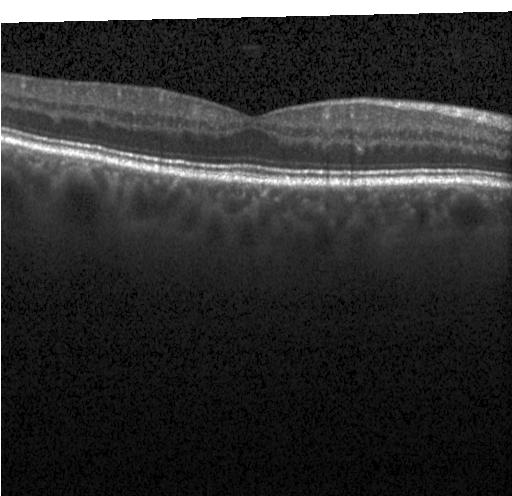

OCT scan showing no evidence of choroidal neovascularization, diabetic macular edema, or drusen.